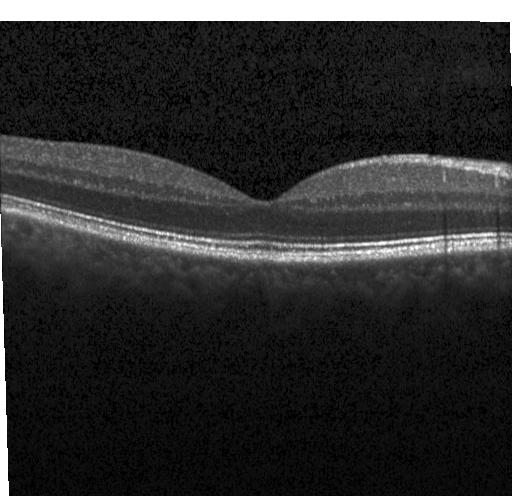
OCT B-scan
This B-scan demonstrates neither choroidal neovascularization, diabetic macular edema, nor drusen.